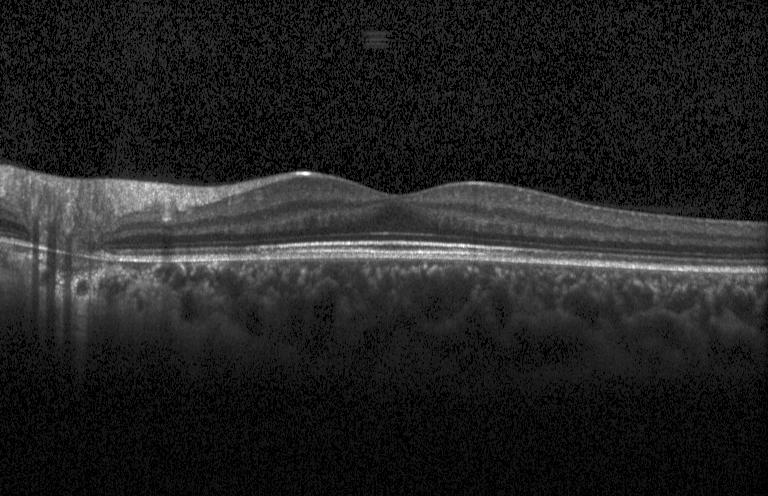

Spectral-domain optical coherence tomography. Retinal OCT cross-section — Dx: no evidence of choroidal neovascularization, diabetic macular edema, or drusen.